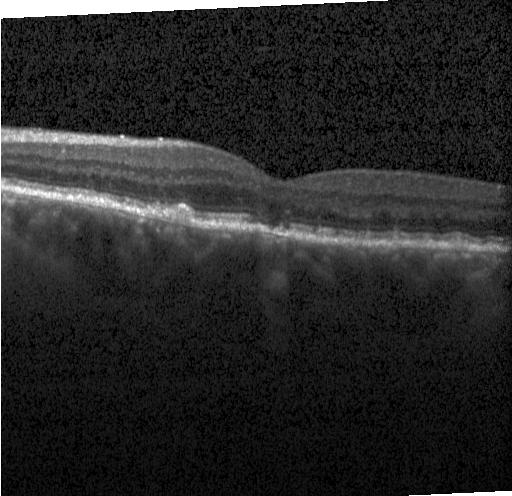
Spectral-domain optical coherence tomography · macular scan · OCT line scan — OCT finding: sub-RPE drusenoid deposits.